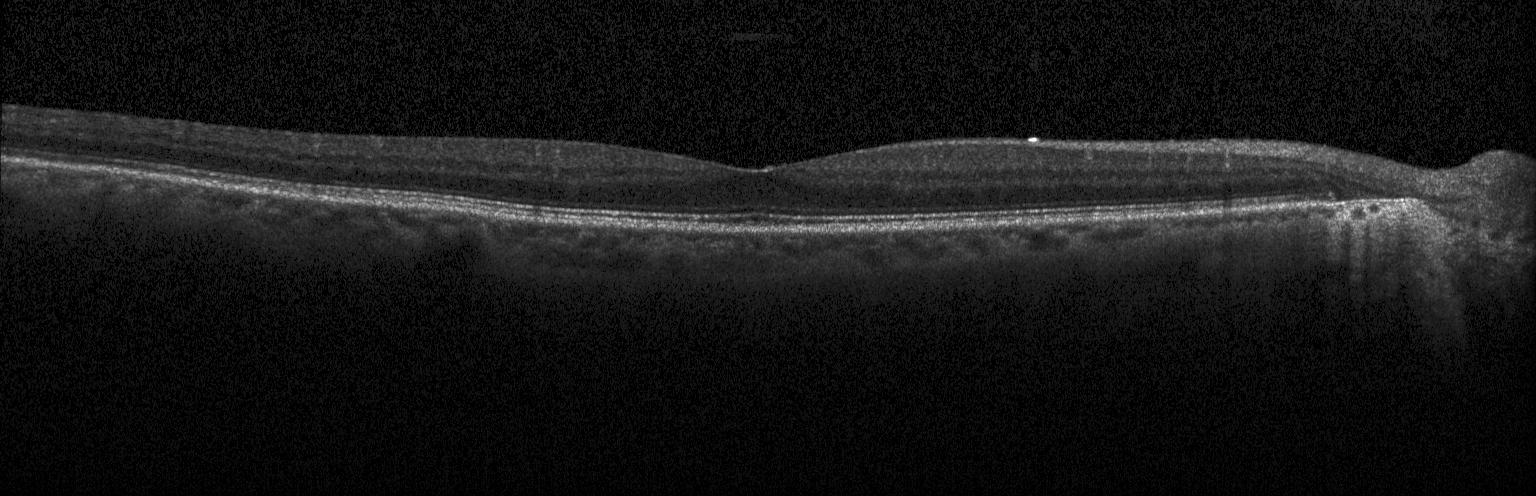

OCT B-scan · Heidelberg Spectralis.
Dx: neither choroidal neovascularization, diabetic macular edema, nor drusen.